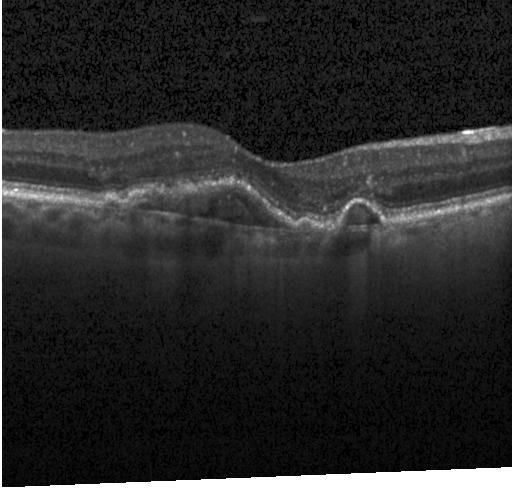
Retinal OCT B-scan.
Diagnosis: CNV.